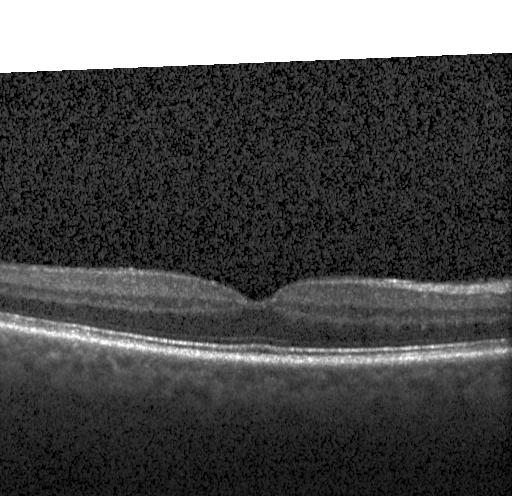 Finding: no CNV, no DME, and no drusen.